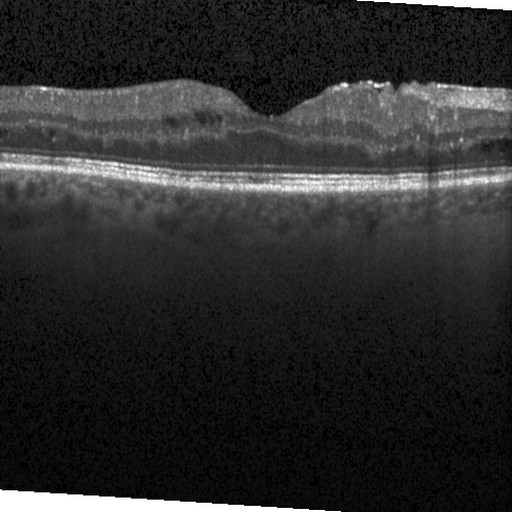

Through the macula · spectral-domain optical coherence tomography · optical coherence tomography B-scan · Heidelberg Spectralis OCT system.
OCT finding: diabetic macular edema.